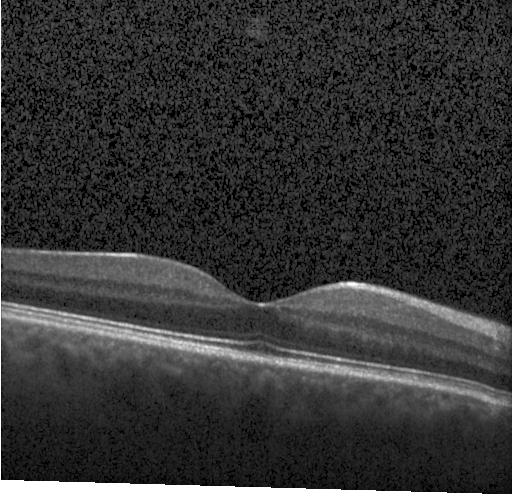 Assessment: neither choroidal neovascularization, diabetic macular edema, nor drusen.